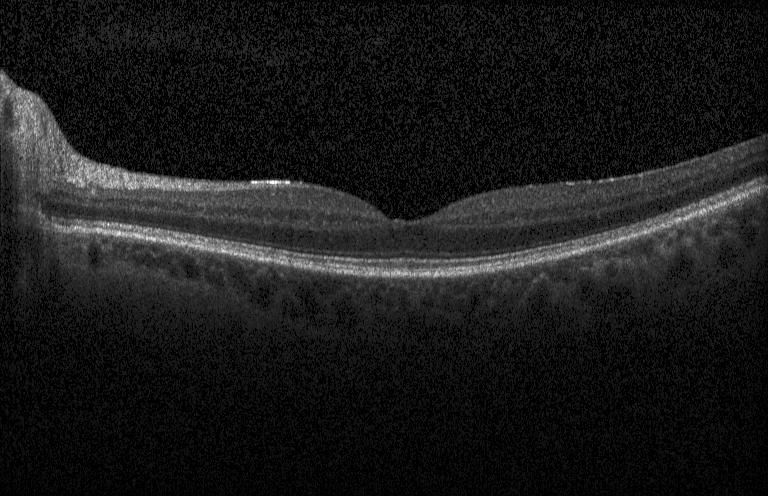
SD-OCT. Centered on the fovea. Optical coherence tomography B-scan. Acquired on a Heidelberg Spectralis
Finding: neither choroidal neovascularization, diabetic macular edema, nor drusen.